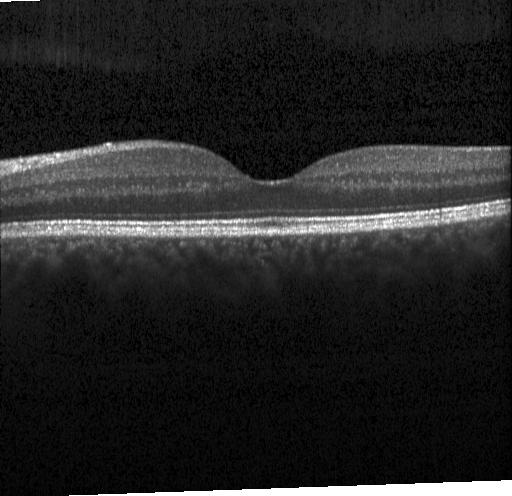
Heidelberg Spectralis. Spectral-domain OCT. Retinal OCT cross-section. Horizontal scan through the fovea.
Neither CNV, DME, nor drusen.